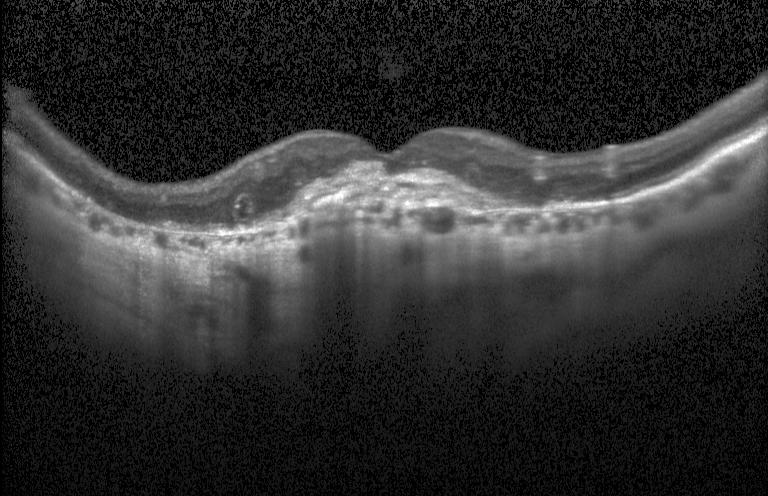 OCT line scan. Dx: CNV.